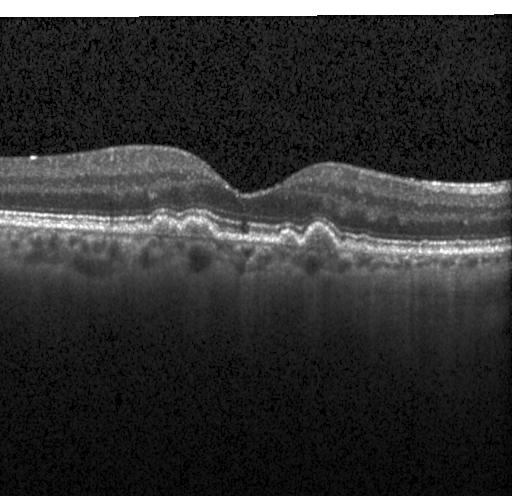
Horizontal scan through the fovea; spectral-domain optical coherence tomography; Heidelberg Spectralis OCT system; optical coherence tomography B-scan. Diagnosis: sub-RPE drusenoid deposits.